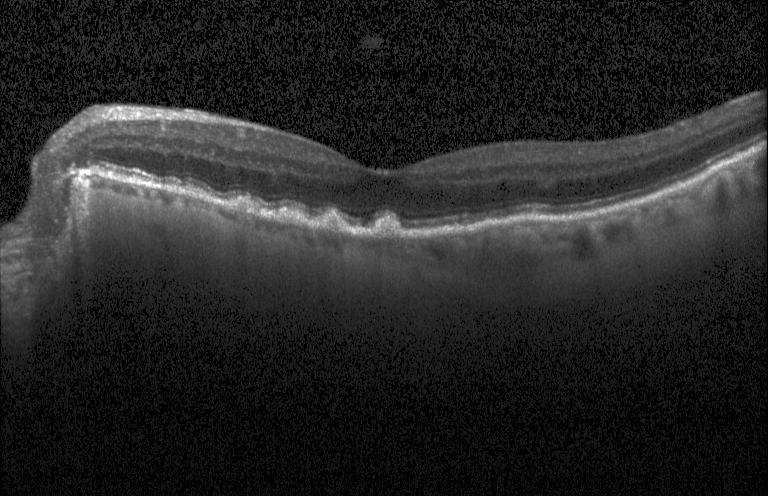 Diagnosis: multiple drusen.